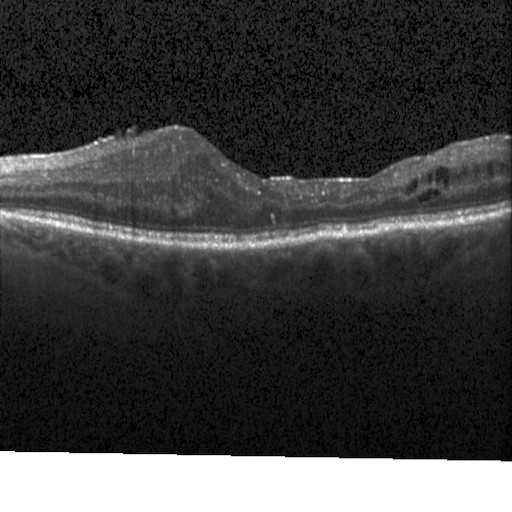

Optical coherence tomography B-scan · Heidelberg Spectralis OCT system · spectral-domain OCT · through the macula. OCT finding: DME.